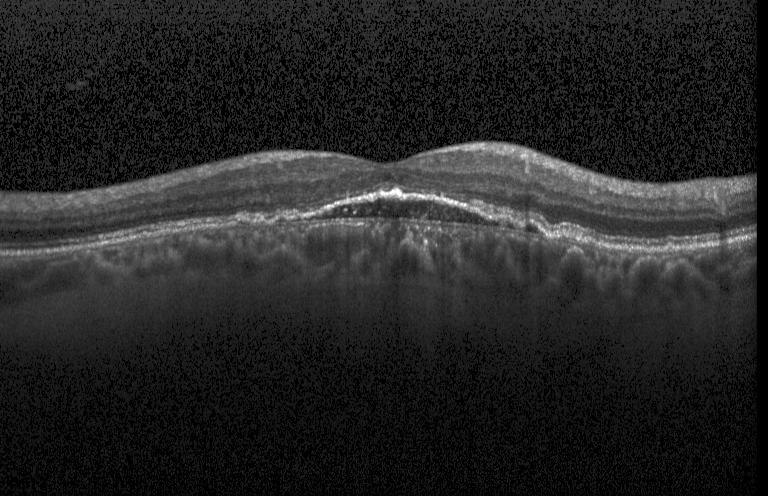
Spectral-domain OCT B-scan: a choroidal neovascular membrane.